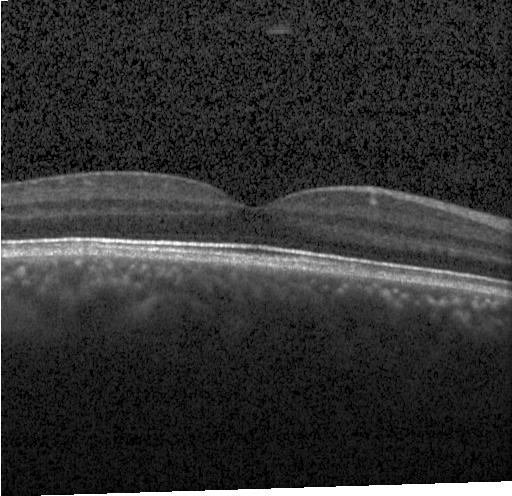
OCT line scan. No evidence of choroidal neovascularization, diabetic macular edema, or drusen.